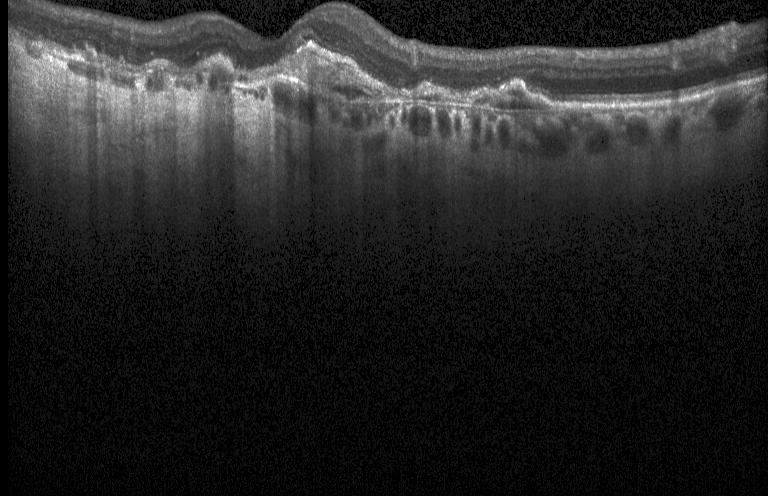 Optical coherence tomography scan.
Diagnosis: a choroidal neovascular membrane.